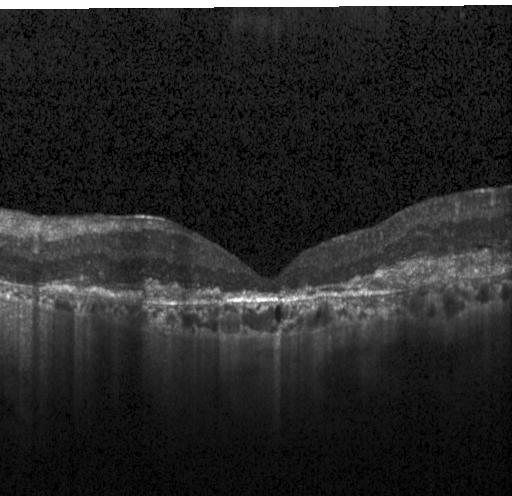 Optical coherence tomography scan.
Impression: CNV.